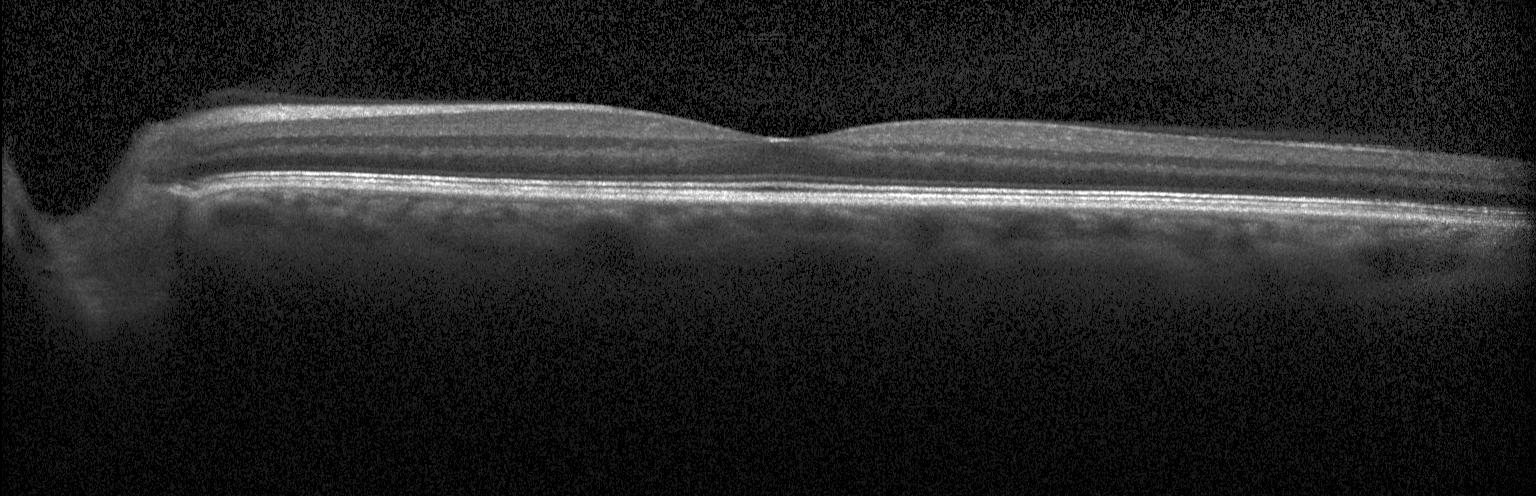 Retinal OCT cross-section showing no choroidal neovascularization, diabetic macular edema, or drusen.